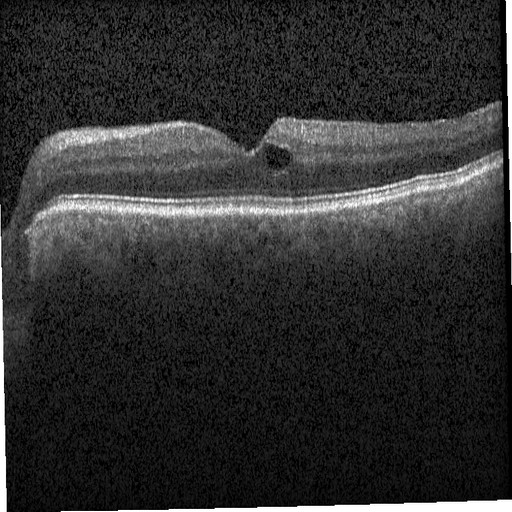

OCT scan showing DME.